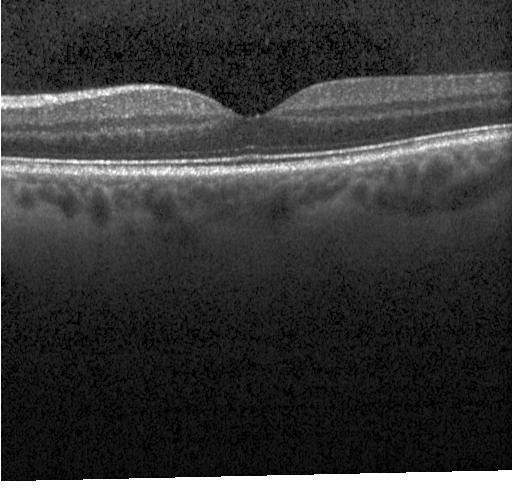 Macular OCT demonstrating neither CNV, DME, nor drusen.